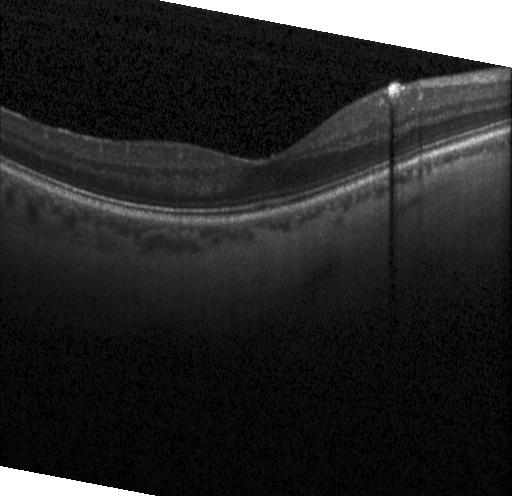 Fovea-centered, retinal OCT cross-section — Macular OCT: no evidence of CNV, DME, or drusen.